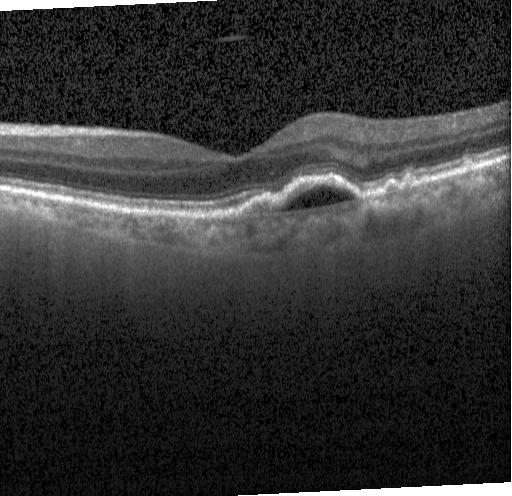 Spectral-domain OCT, retinal OCT B-scan, centered on the fovea, Heidelberg Spectralis
Diagnosis: a choroidal neovascular membrane.